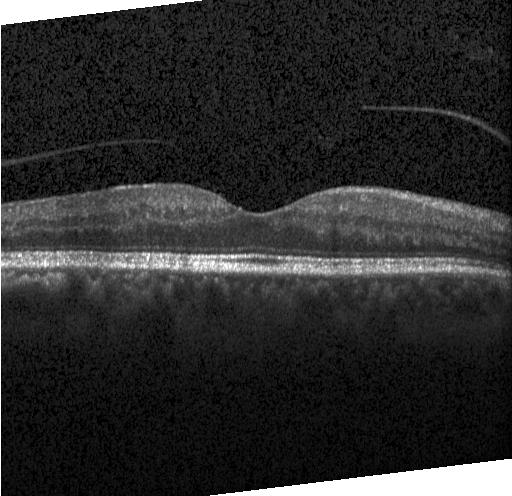

Optical coherence tomography B-scan. Impression: no choroidal neovascularization, diabetic macular edema, or drusen.